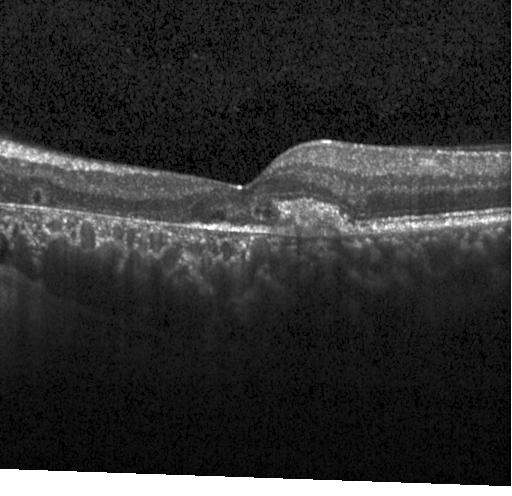

Retinal OCT cross-section, spectral-domain optical coherence tomography, centered on the fovea, acquired on a Heidelberg Spectralis.
Impression: choroidal neovascularization.